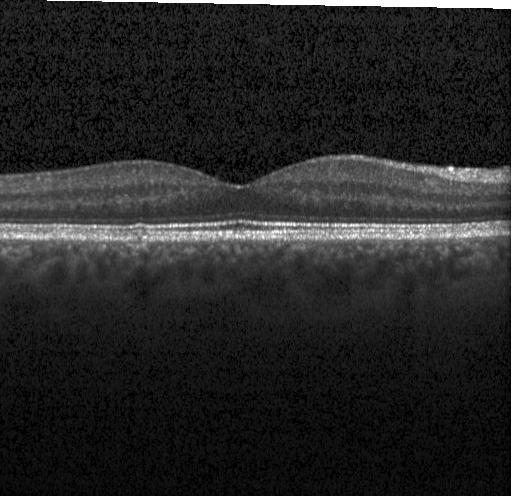

Retinal OCT cross-section.
Neither choroidal neovascularization, diabetic macular edema, nor drusen.